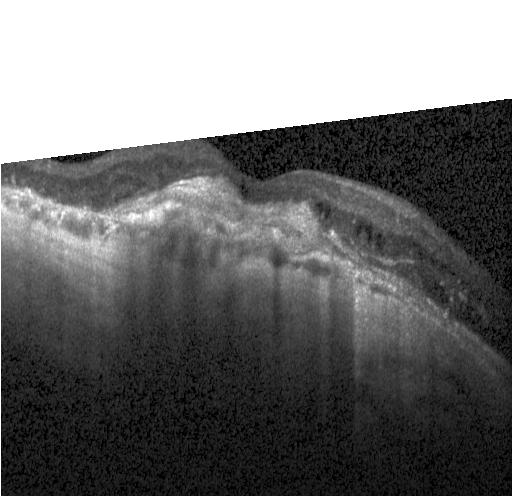

OCT finding: a choroidal neovascular membrane.